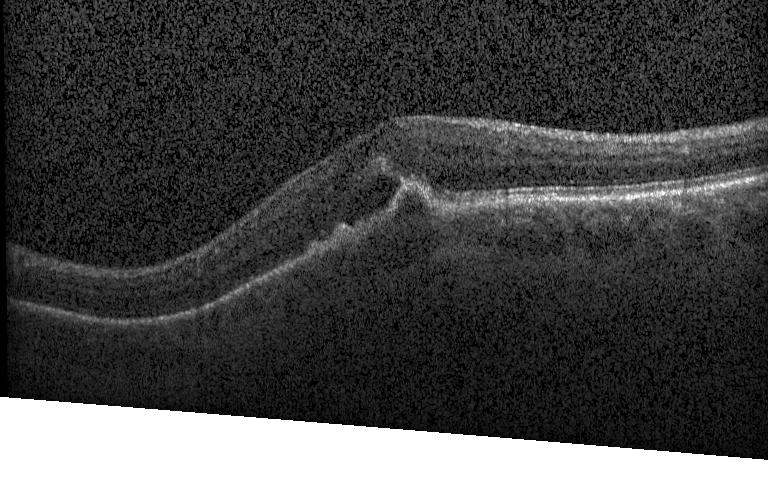

Retinal OCT B-scan
Finding: CNV.